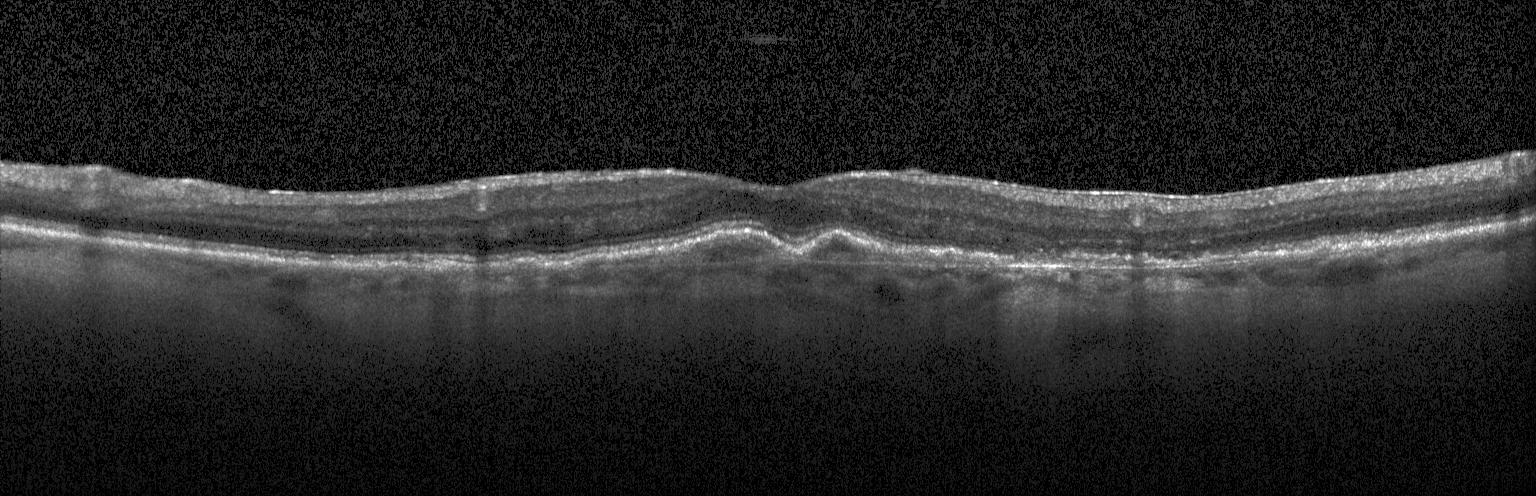
Fovea-centered. Acquired on a Heidelberg Spectralis. Optical coherence tomography scan. Spectral-domain optical coherence tomography.
Impression: a choroidal neovascular membrane.